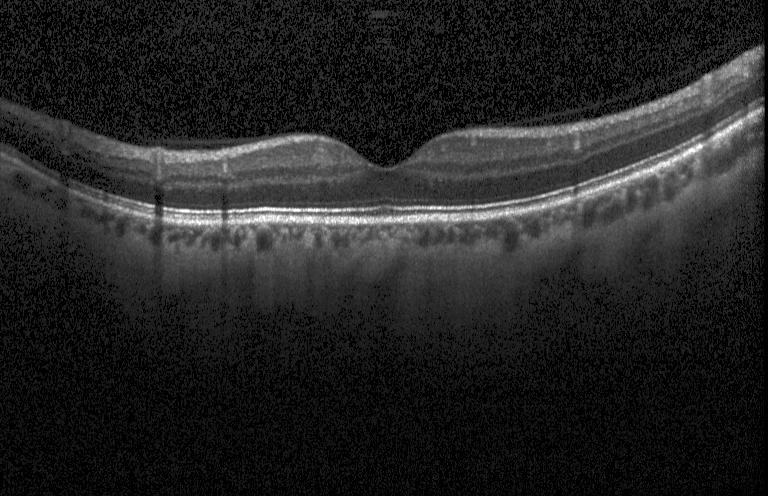

Macular OCT: no choroidal neovascularization, no diabetic macular edema, and no drusen.